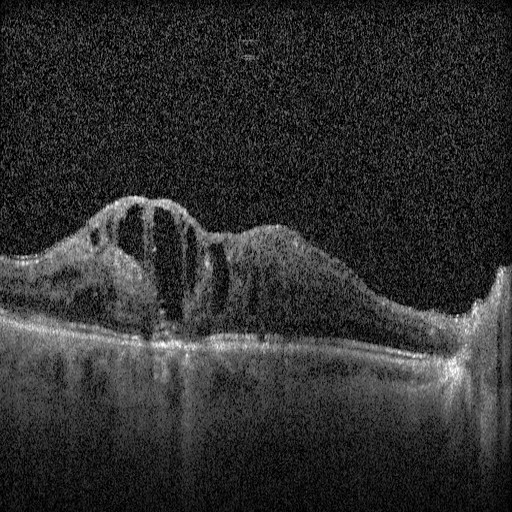 The scan shows DME.